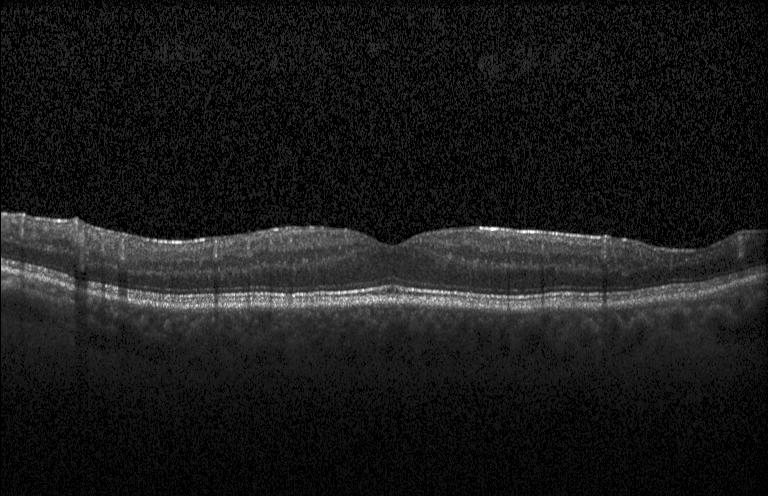 Through the macula · OCT line scan — The scan shows neither choroidal neovascularization, diabetic macular edema, nor drusen.